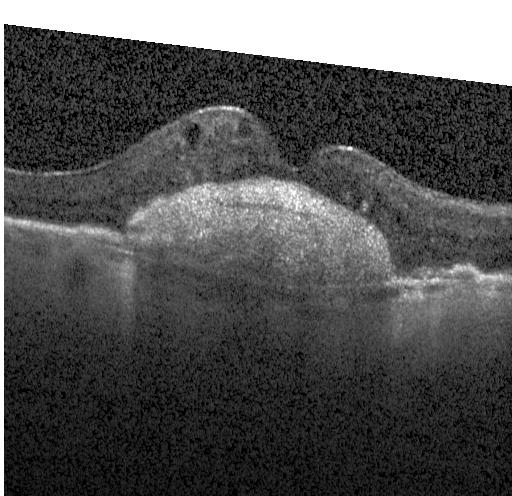
Heidelberg Spectralis. OCT line scan.
Assessment: a choroidal neovascular membrane.